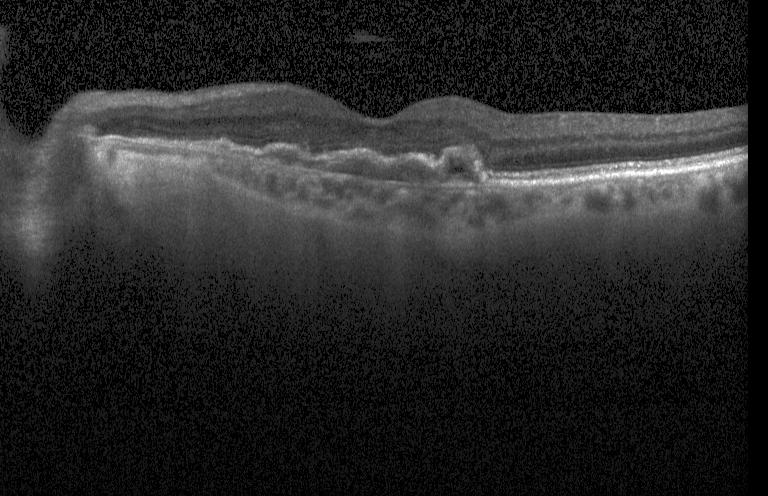
Assessment: a choroidal neovascular membrane.